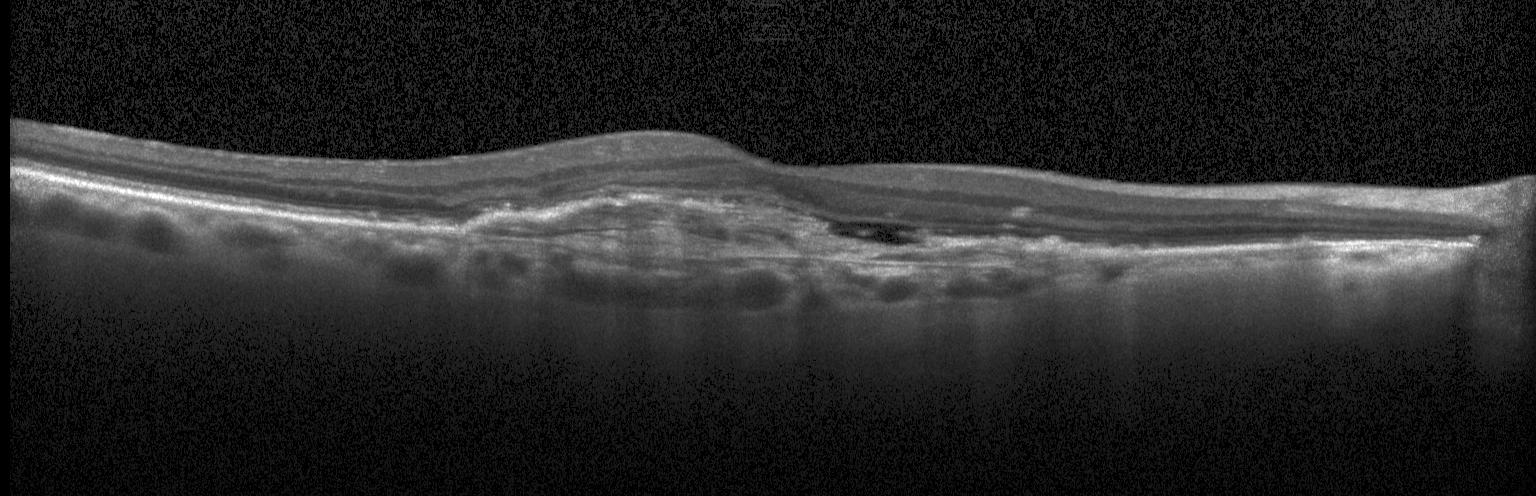 Finding: CNV.